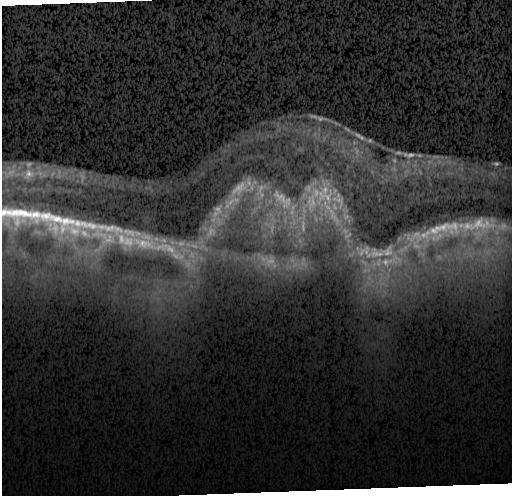

SD-OCT · optical coherence tomography B-scan — Impression: a choroidal neovascular membrane.